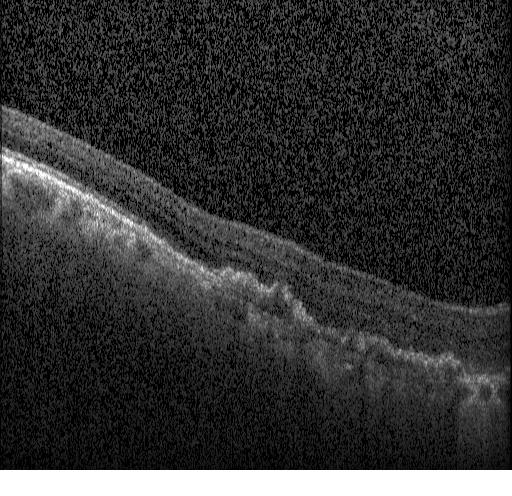
Macular OCT: choroidal neovascularization (CNV).